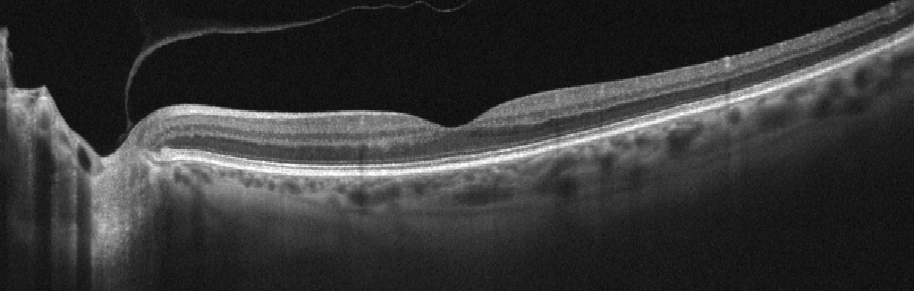
Oculus dexter; OCT B-scan; instrument: Optovue Avanti RTVue XR; fovea-centered.
The scan shows no AMD, DME, ERM, RAO, RVO, or VID.